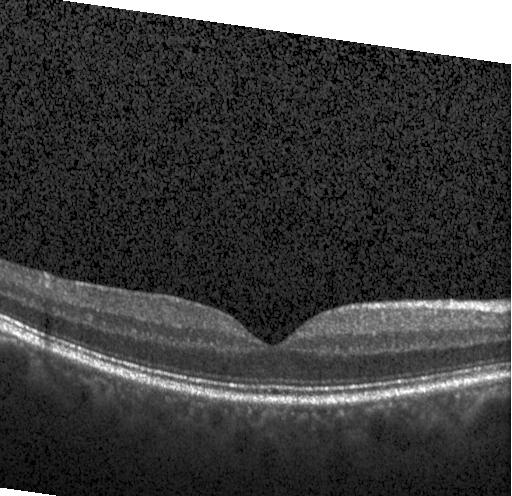

OCT B-scan
Macular OCT: no choroidal neovascularization, diabetic macular edema, or drusen.